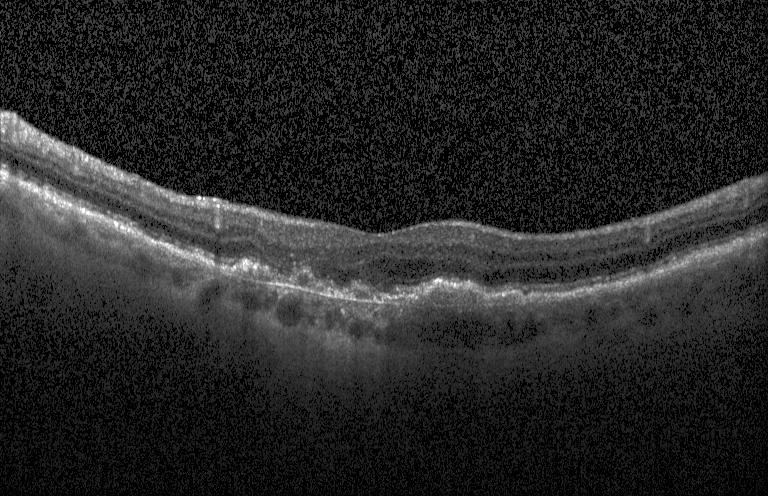 Acquired on a Heidelberg Spectralis. Retinal OCT B-scan. Through the macula — The scan shows CNV.